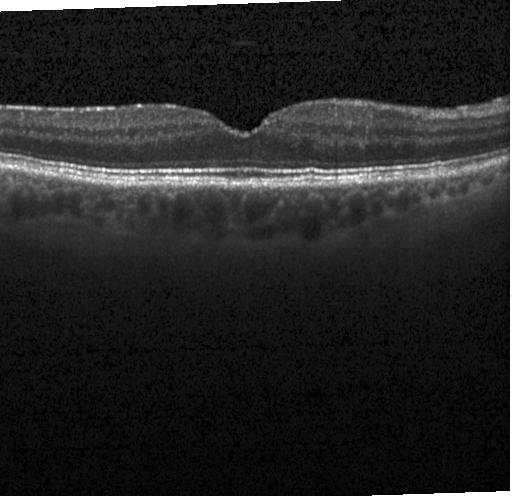

Impression: no choroidal neovascularization, diabetic macular edema, or drusen.